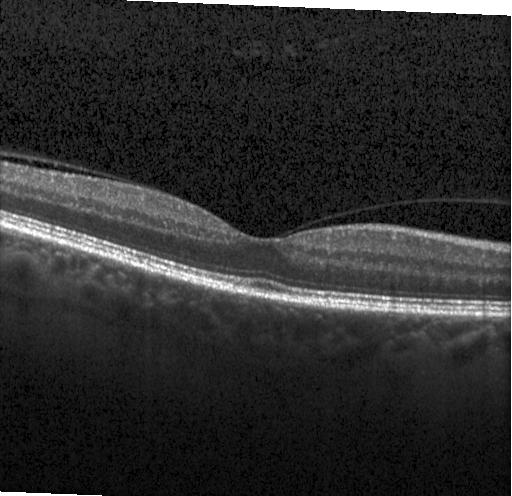 Retinal OCT B-scan; acquired on a Heidelberg Spectralis; SD-OCT
Diagnosis: no CNV, DME, or drusen.